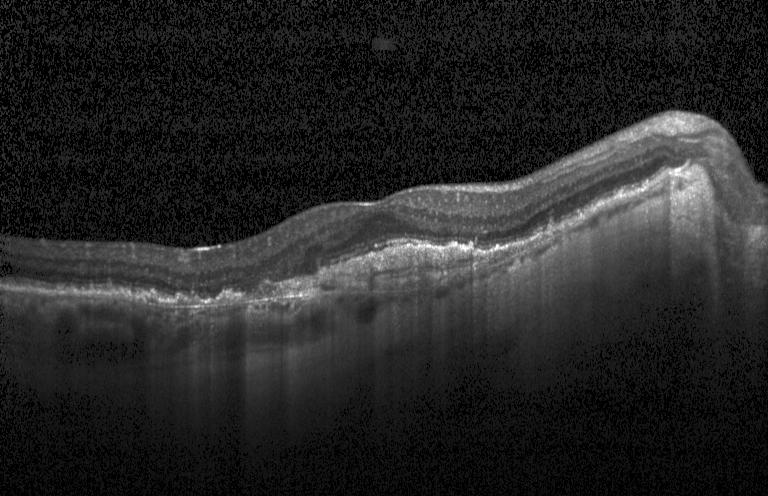
OCT scan showing choroidal neovascularization.